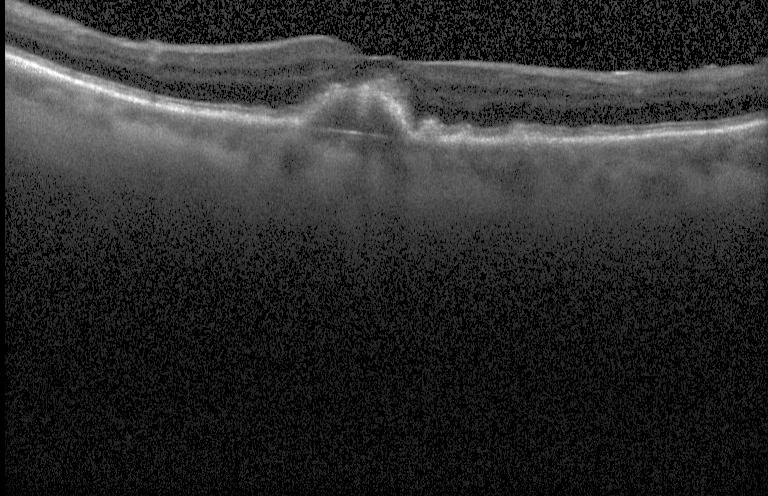
Macular OCT: a choroidal neovascular membrane.